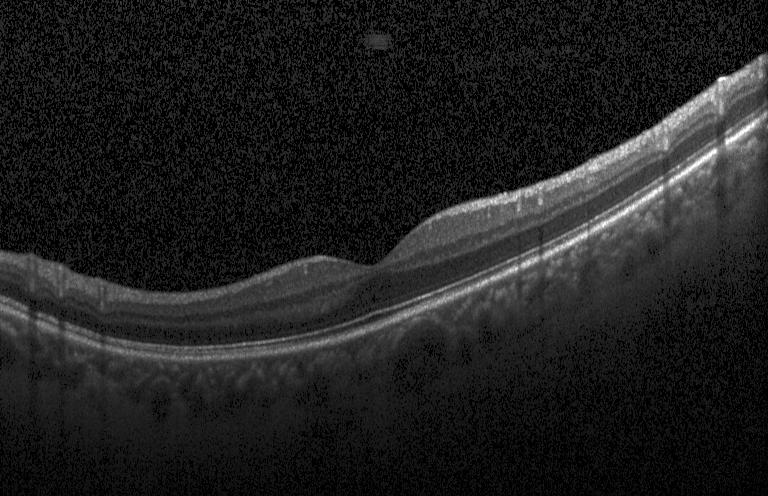 Heidelberg Spectralis, SD-OCT, through the macula, OCT line scan.
No CNV, no DME, and no drusen.